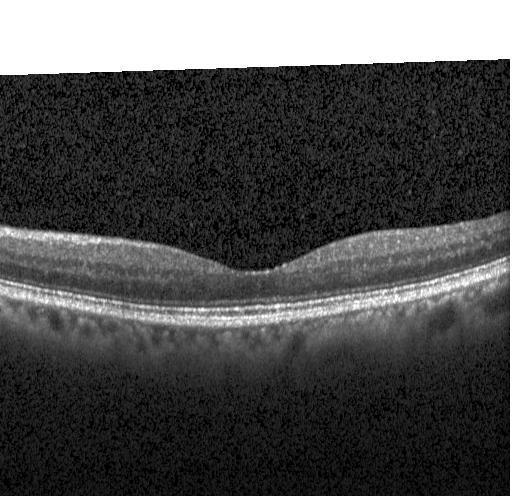 Retinal OCT B-scan.
Impression: no choroidal neovascularization, no diabetic macular edema, and no drusen.